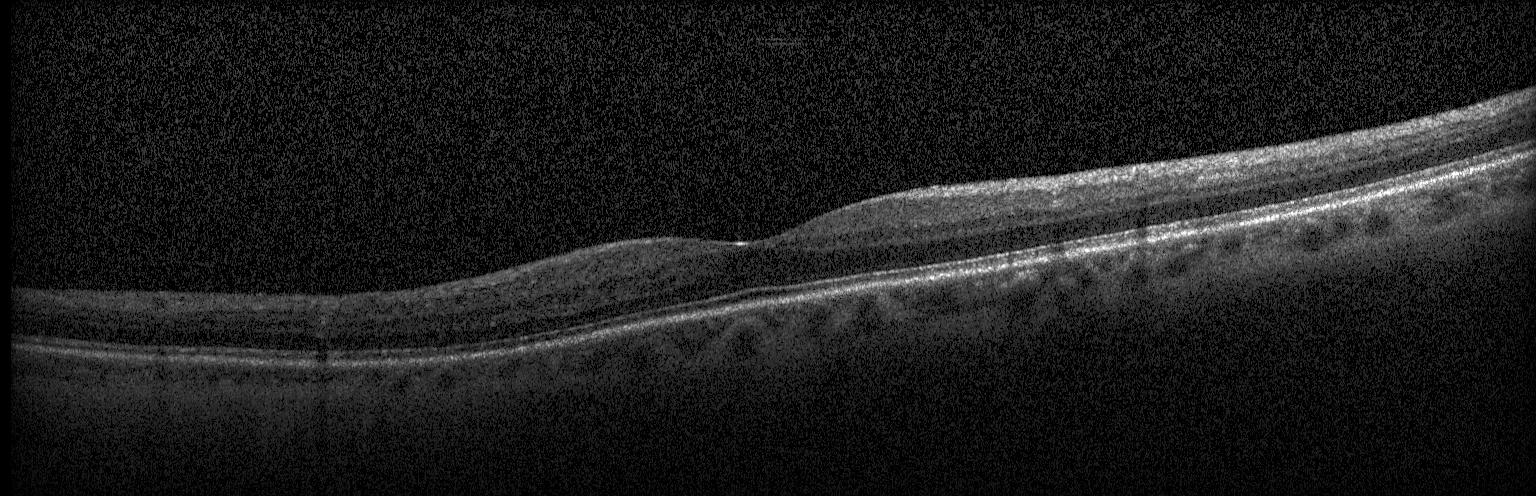
Horizontal scan through the fovea. Optical coherence tomography B-scan. Spectral-domain optical coherence tomography. Instrument: Heidelberg Spectralis
Diagnosis: neither CNV, DME, nor drusen.